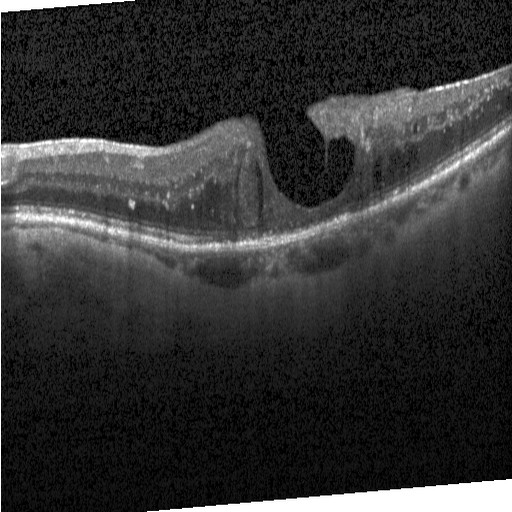 Finding: diabetic macular edema (DME).